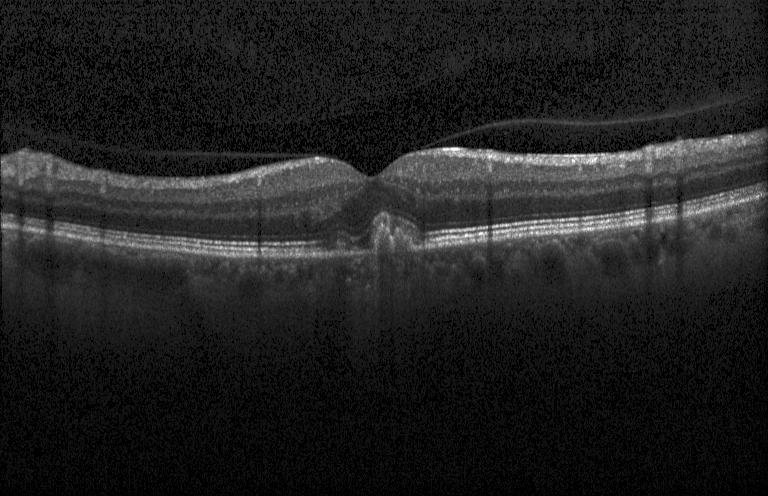

Diagnosis: drusen.